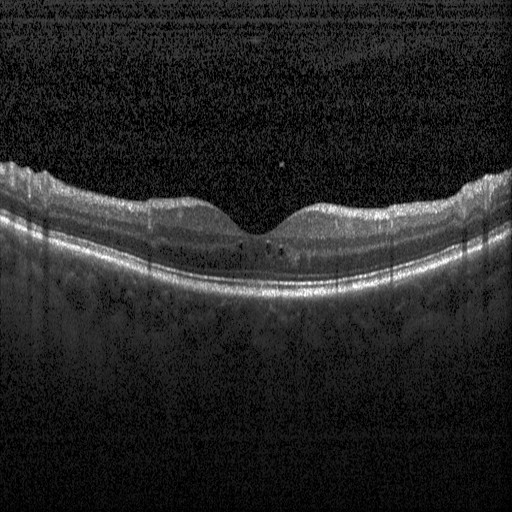

Instrument: Heidelberg Spectralis. Through the macula. Retinal OCT B-scan. Spectral-domain OCT — Impression: diabetic macular edema (DME).